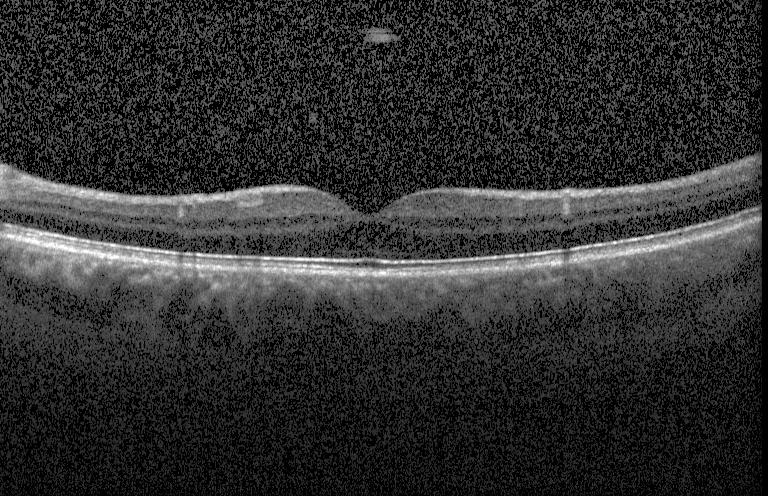

Optical coherence tomography B-scan. Assessment: no choroidal neovascularization, no diabetic macular edema, and no drusen.